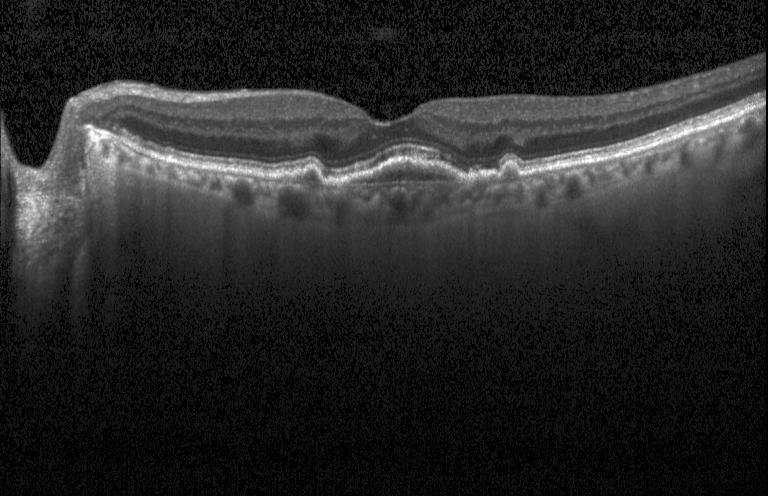
Diagnosis: CNV.